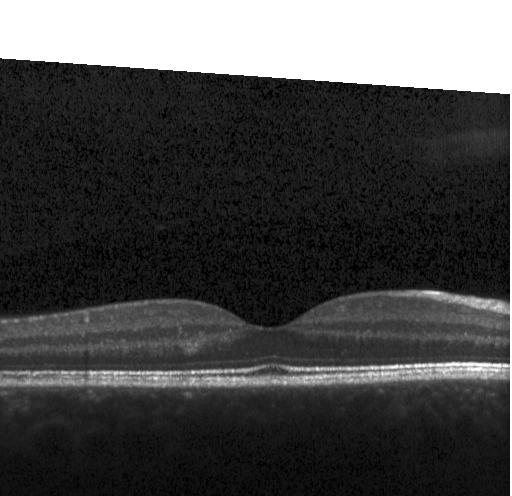

Heidelberg Spectralis, optical coherence tomography scan, through the macula. Assessment: no evidence of choroidal neovascularization, diabetic macular edema, or drusen.